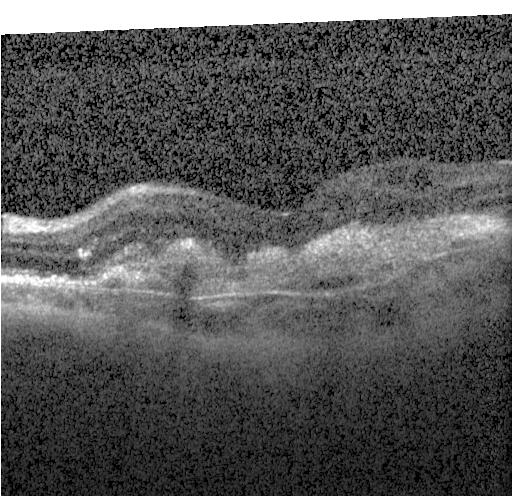 Spectral-domain OCT; retinal OCT B-scan; fovea-centered. Finding: choroidal neovascularization (CNV).